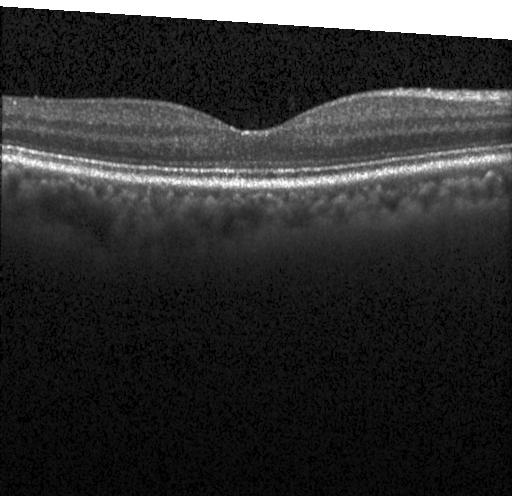 Optical coherence tomography scan; centered on the fovea. This B-scan demonstrates no choroidal neovascularization, diabetic macular edema, or drusen.